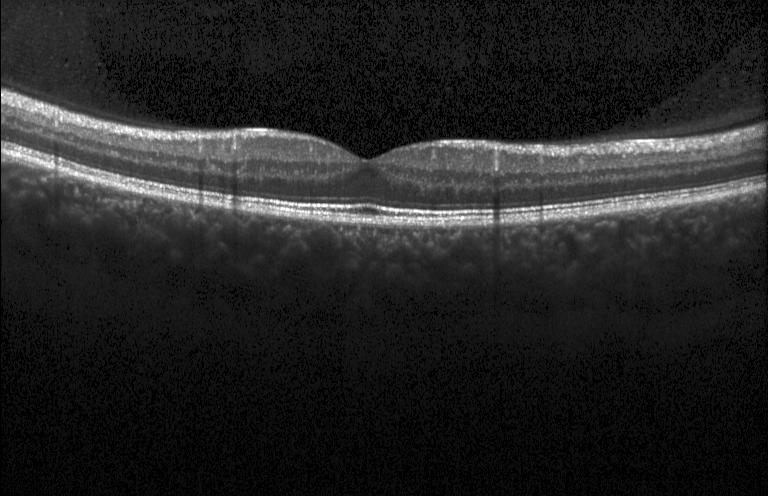

The scan shows no choroidal neovascularization, no diabetic macular edema, and no drusen.